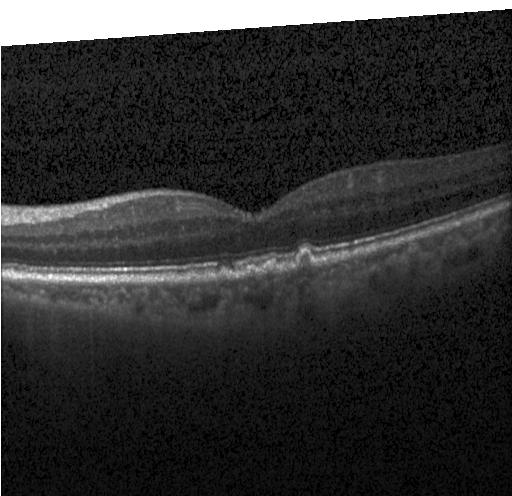
Macular OCT: drusen.